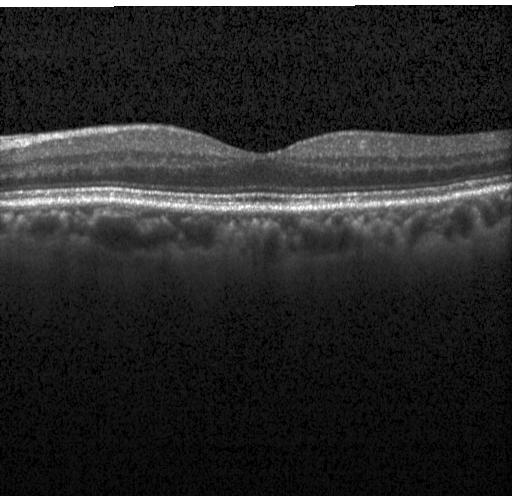
Spectral-domain OCT · instrument: Heidelberg Spectralis · macular scan · OCT line scan — This B-scan demonstrates no evidence of choroidal neovascularization, diabetic macular edema, or drusen.